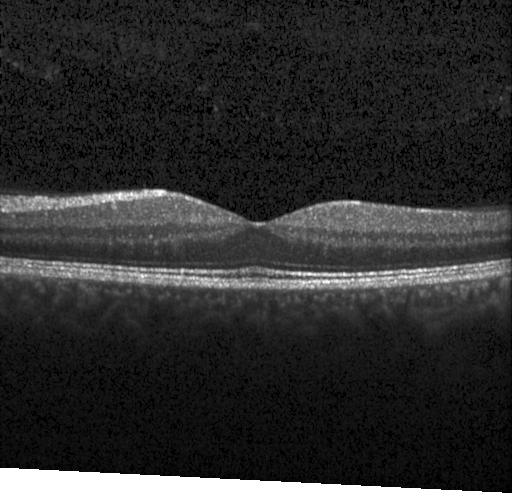

Retinal OCT B-scan.
Macular OCT: no evidence of choroidal neovascularization, diabetic macular edema, or drusen.